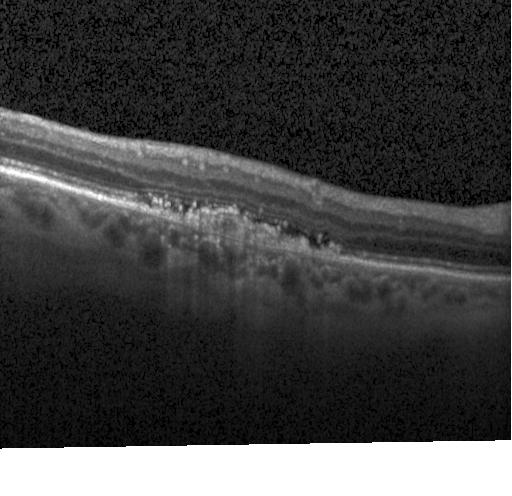 Retinal OCT B-scan.
Choroidal neovascularization.